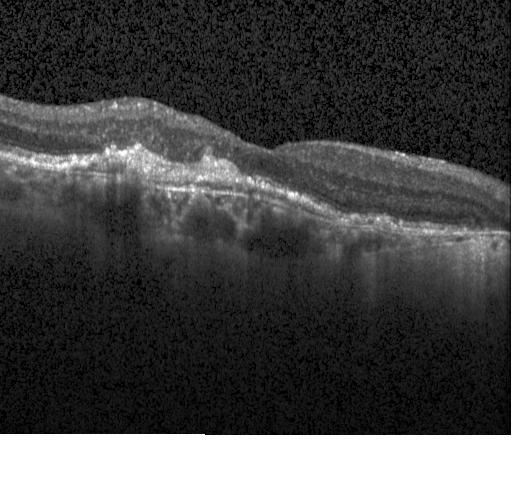
OCT finding: a choroidal neovascular membrane.